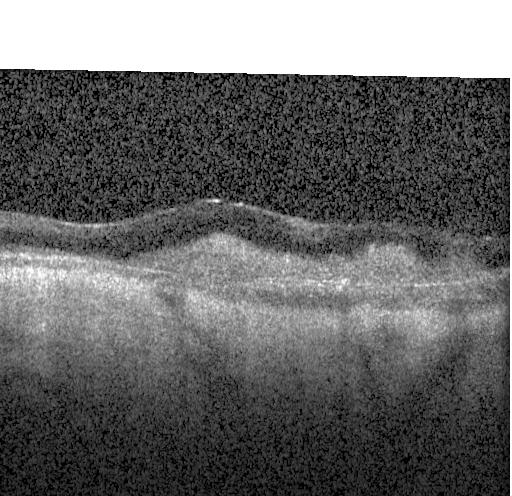

Retinal OCT cross-section, centered on the fovea — Diagnosis: choroidal neovascularization.